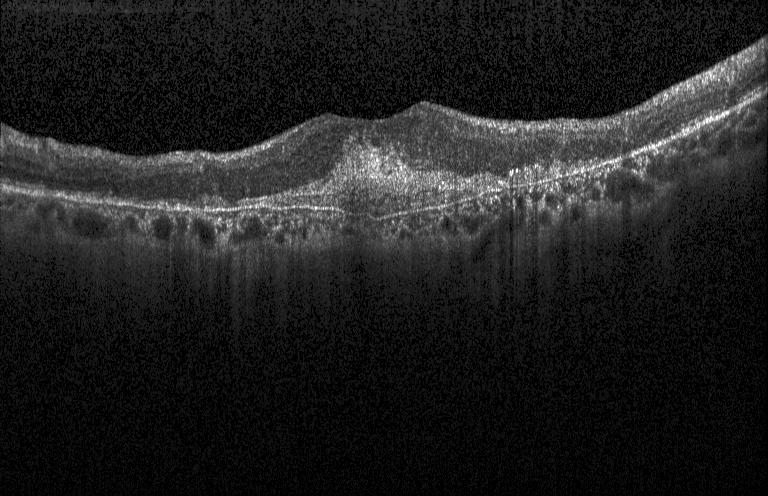
Diagnosis: choroidal neovascularization (CNV).